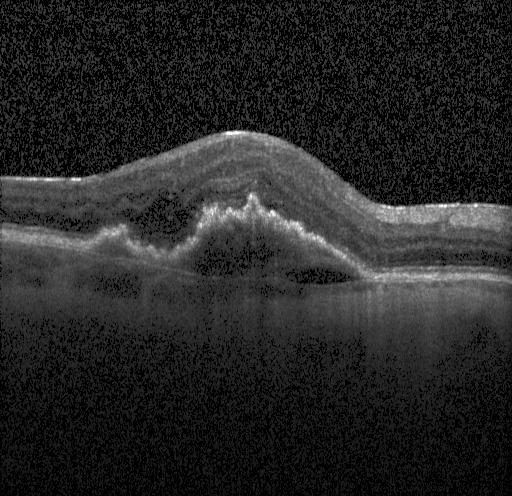 OCT finding: a choroidal neovascular membrane.